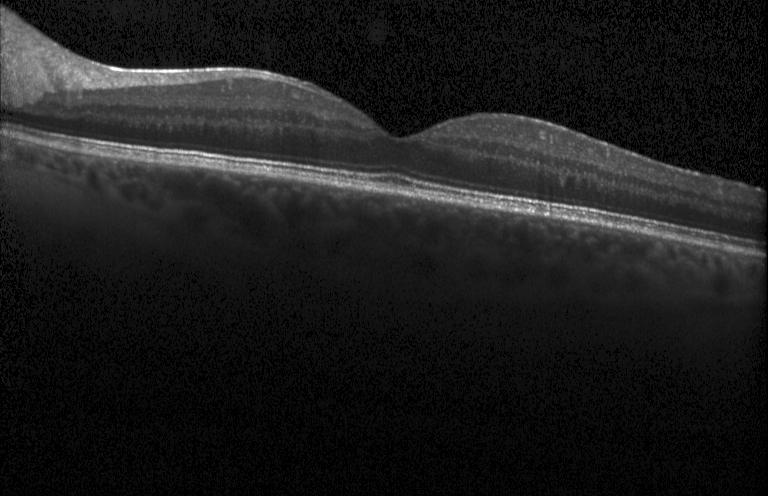

Heidelberg Spectralis OCT system. OCT line scan. Spectral-domain optical coherence tomography — Neither choroidal neovascularization, diabetic macular edema, nor drusen.